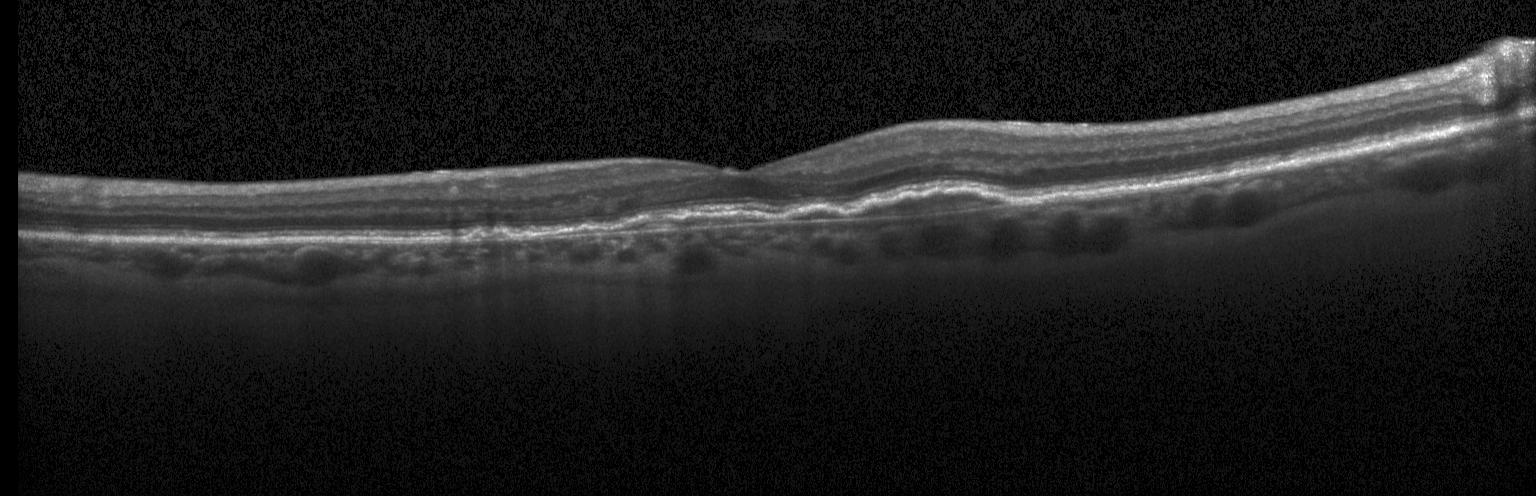
Heidelberg Spectralis OCT system. Optical coherence tomography scan. Dx: a choroidal neovascular membrane.